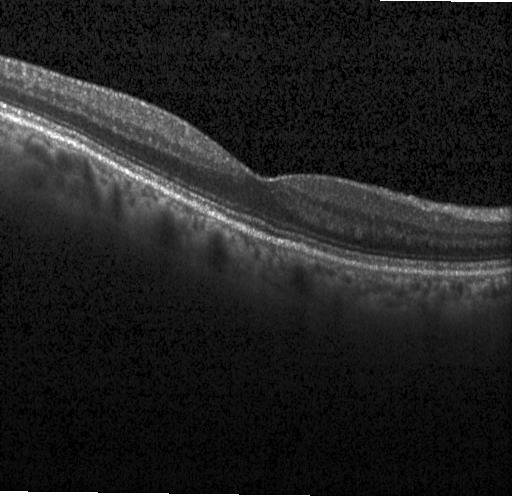

Finding: no evidence of CNV, DME, or drusen.